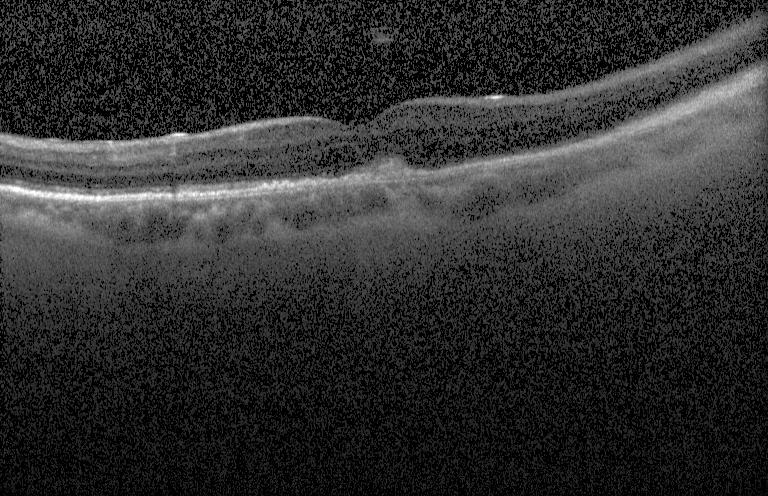
Retinal OCT cross-section showing choroidal neovascularization (CNV).